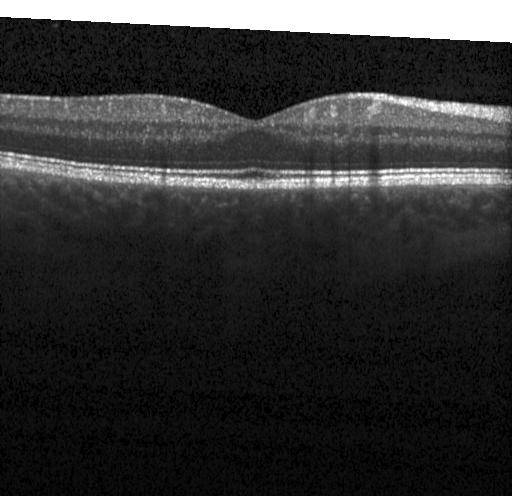 Heidelberg Spectralis OCT system. Optical coherence tomography B-scan
Finding: no choroidal neovascularization, diabetic macular edema, or drusen.